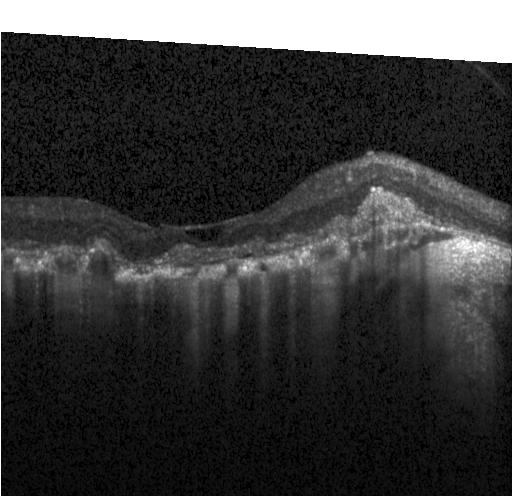
OCT finding: a choroidal neovascular membrane.